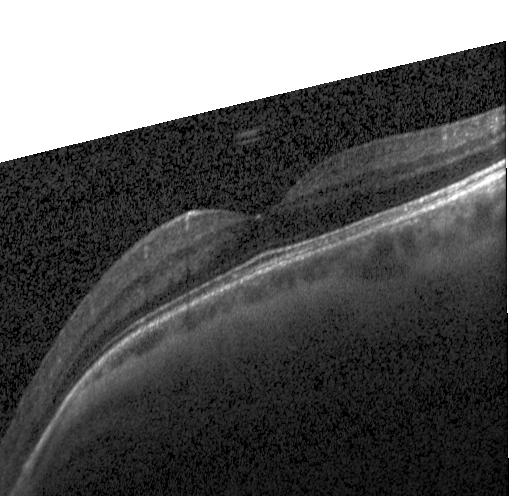
OCT B-scan. SD-OCT. Through the macula. Instrument: Heidelberg Spectralis
Assessment: no choroidal neovascularization, no diabetic macular edema, and no drusen.